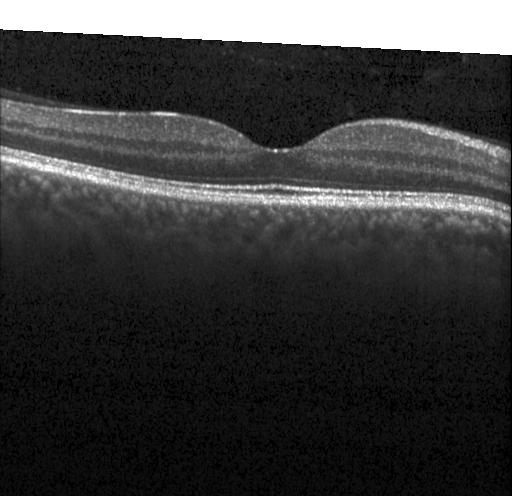

OCT finding: no CNV, DME, or drusen.